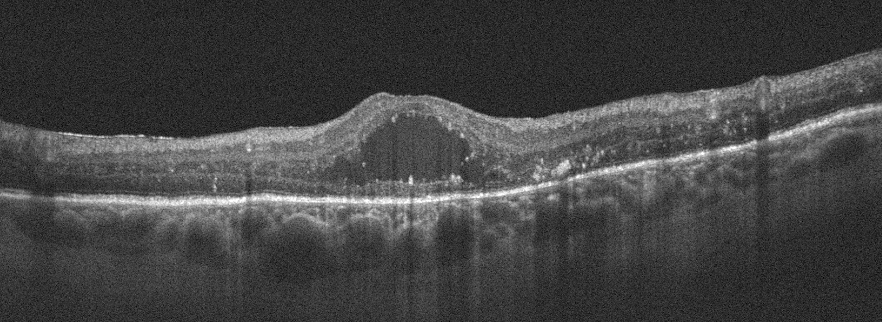

Macular scan; retinal OCT B-scan — Assessment: DME.